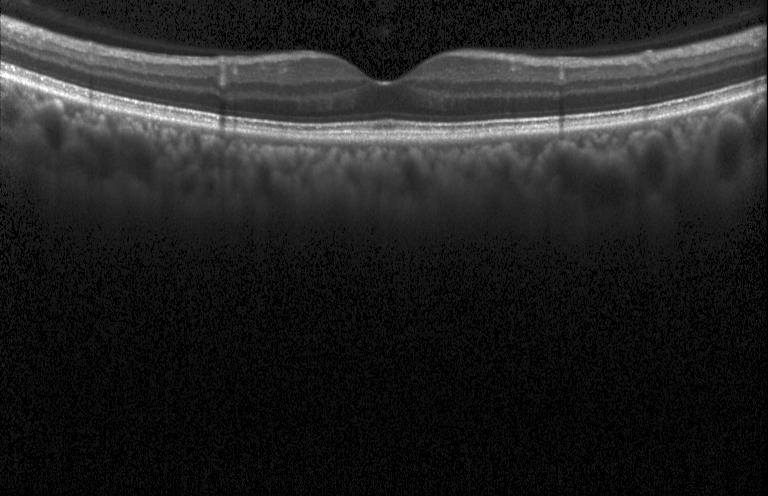

Impression: no CNV, DME, or drusen.